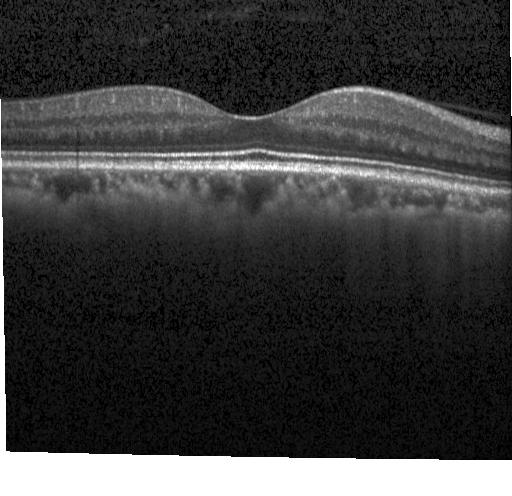

Assessment: neither CNV, DME, nor drusen.